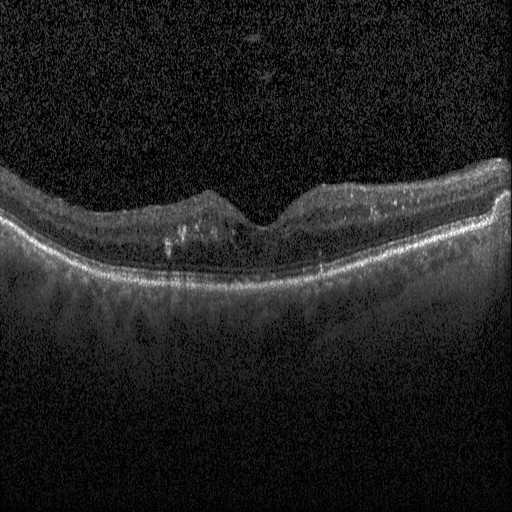
Macular scan · SD-OCT · optical coherence tomography scan · acquired on a Heidelberg Spectralis — Diagnosis: DME.